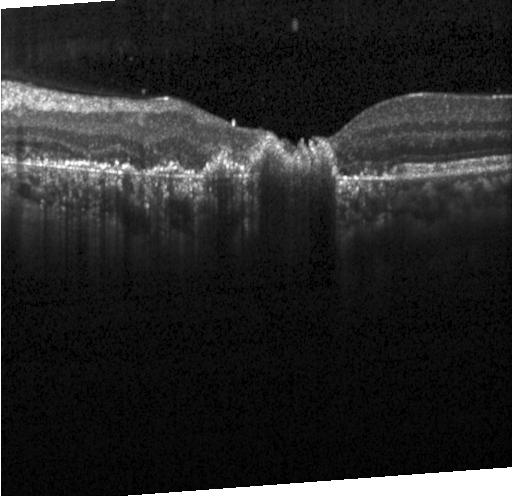

OCT B-scan.
Finding: choroidal neovascularization (CNV).